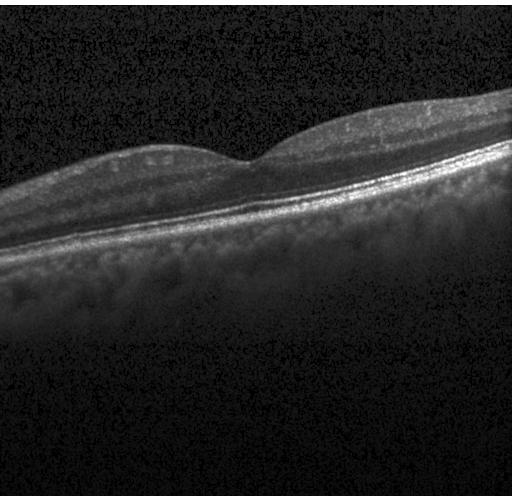 Macular OCT: no choroidal neovascularization, no diabetic macular edema, and no drusen.